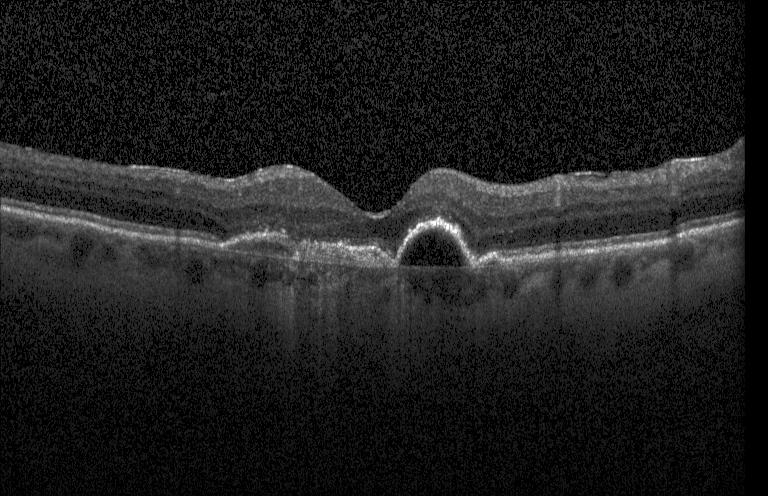
Centered on the fovea; Heidelberg Spectralis OCT system; SD-OCT; retinal OCT cross-section — A choroidal neovascular membrane.